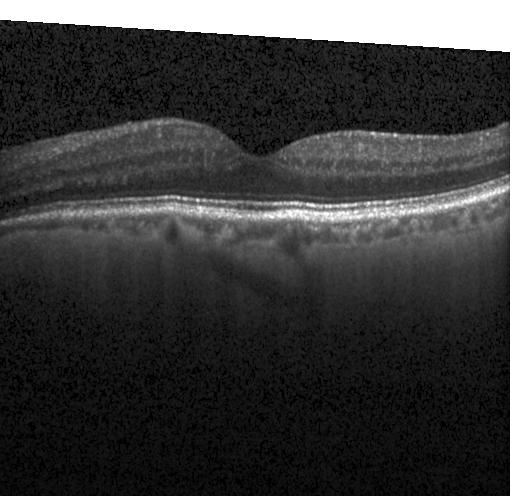

OCT B-scan. Diagnosis: neither choroidal neovascularization, diabetic macular edema, nor drusen.